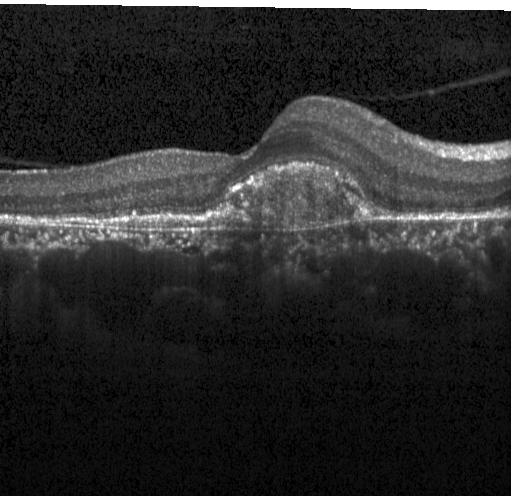
Optical coherence tomography scan; instrument: Heidelberg Spectralis.
Dx: a choroidal neovascular membrane.